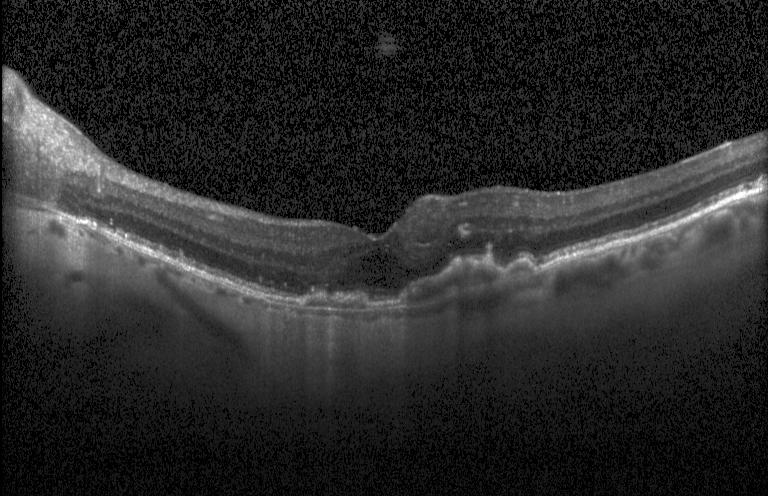 Horizontal scan through the fovea; OCT line scan; instrument: Heidelberg Spectralis — Assessment: choroidal neovascularization.